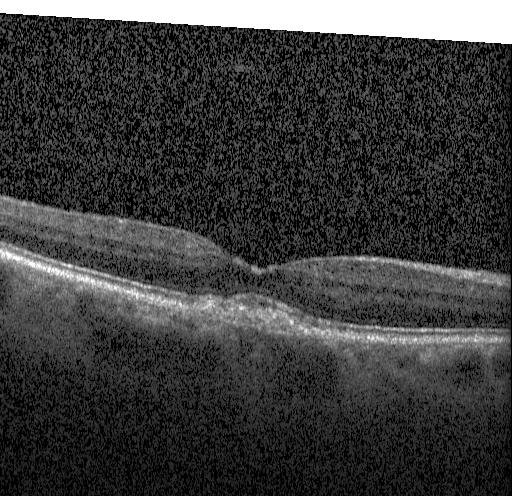 Macular OCT: multiple drusen.